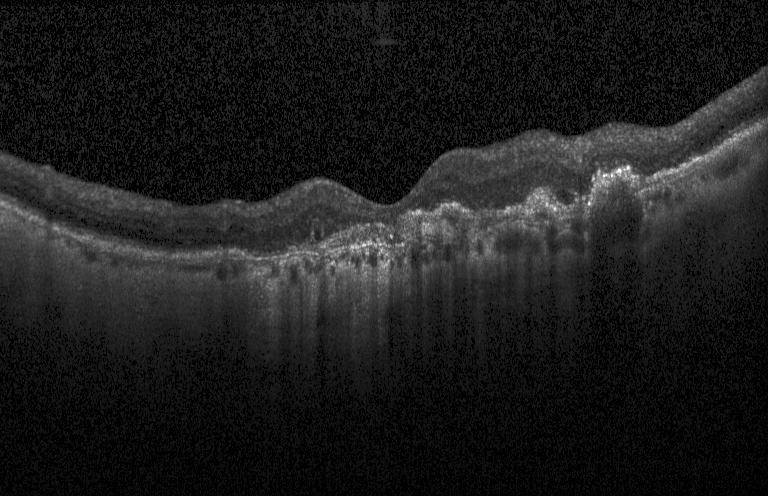

Macular scan, OCT B-scan, Heidelberg Spectralis — Finding: a choroidal neovascular membrane.